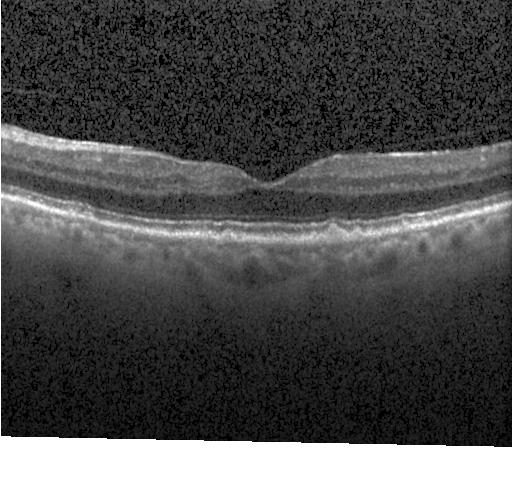 Through the macula; Heidelberg Spectralis; retinal OCT B-scan.
Finding: sub-RPE drusenoid deposits.